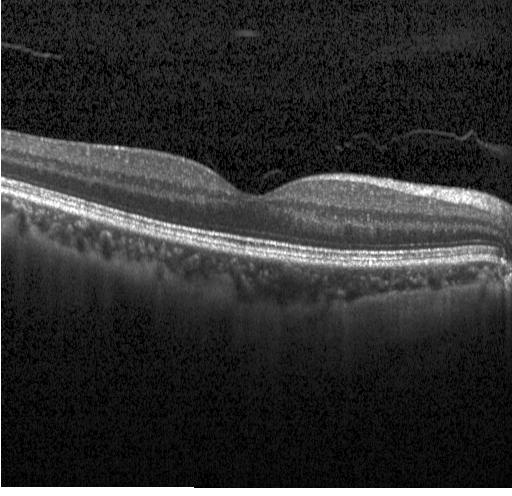

SD-OCT; OCT line scan; instrument: Heidelberg Spectralis; through the macula.
Impression: no evidence of choroidal neovascularization, diabetic macular edema, or drusen.